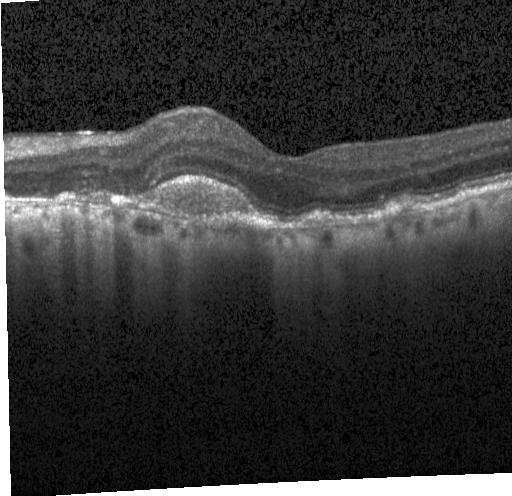

Spectral-domain OCT B-scan: a choroidal neovascular membrane.